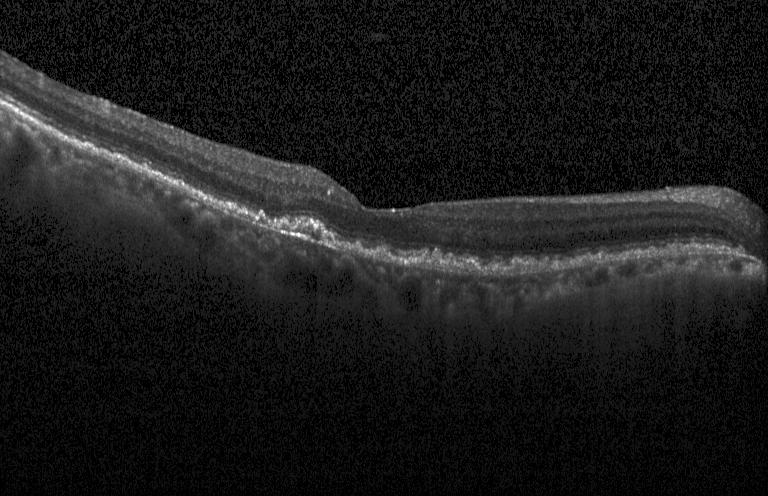
Optical coherence tomography scan; macular scan — Macular OCT: a choroidal neovascular membrane.